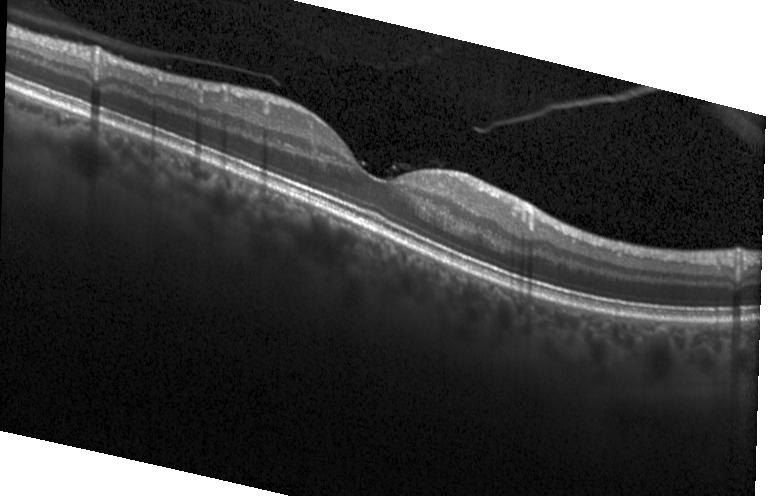

Heidelberg Spectralis OCT system; OCT B-scan
The scan shows no choroidal neovascularization, diabetic macular edema, or drusen.